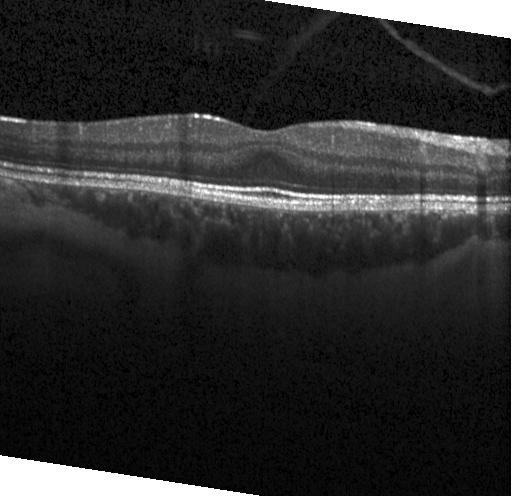

Macular OCT: no evidence of choroidal neovascularization, diabetic macular edema, or drusen.